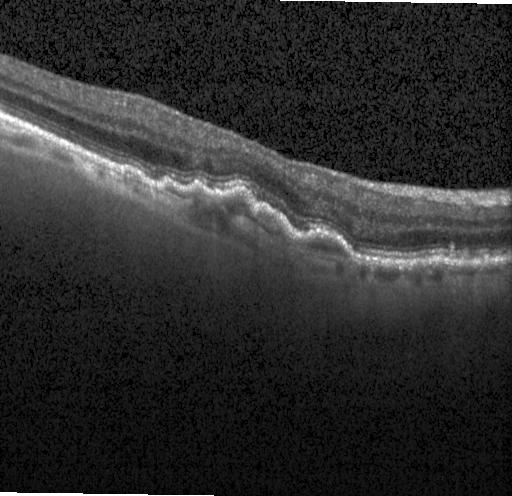
Dx: choroidal neovascularization (CNV).